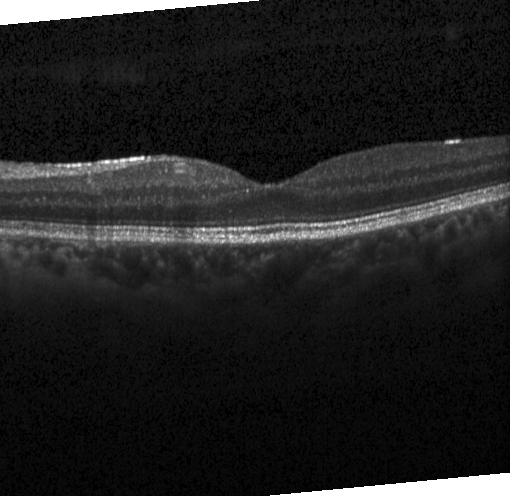
Heidelberg Spectralis OCT system, retinal OCT cross-section, through the macula. Assessment: no evidence of choroidal neovascularization, diabetic macular edema, or drusen.